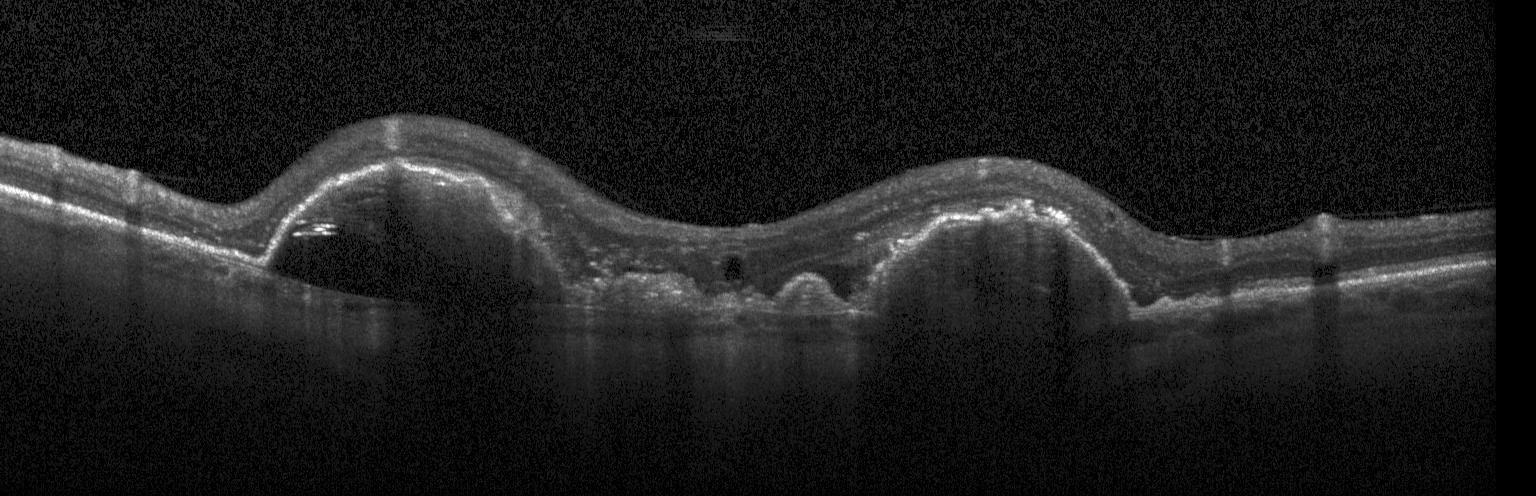 Spectral-domain OCT. Optical coherence tomography scan. Heidelberg Spectralis OCT system — Finding: a choroidal neovascular membrane.